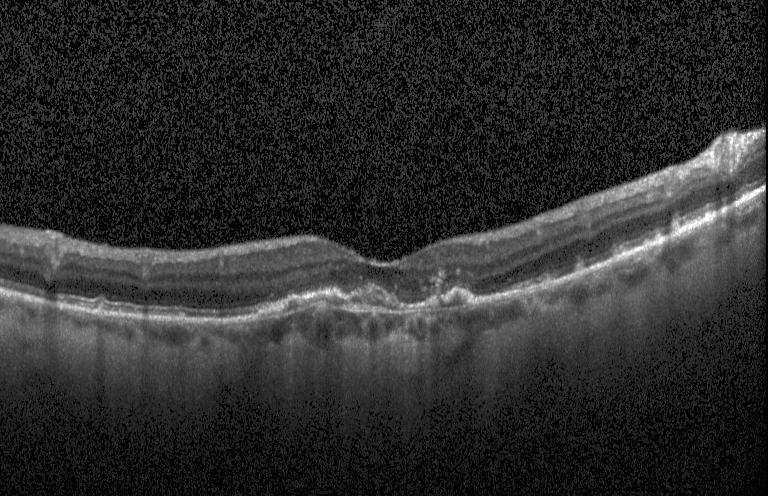
Retinal OCT B-scan — Assessment: a choroidal neovascular membrane.